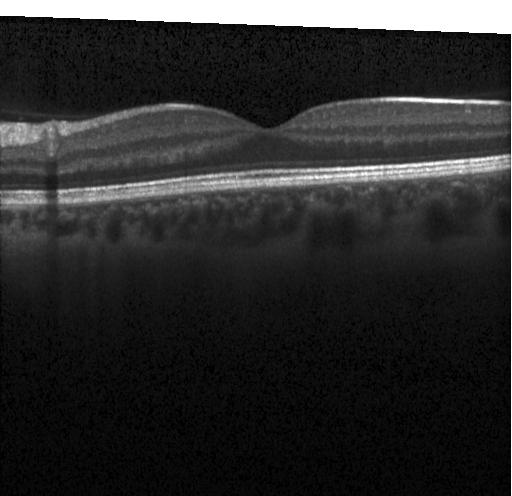
Finding: no choroidal neovascularization, diabetic macular edema, or drusen.